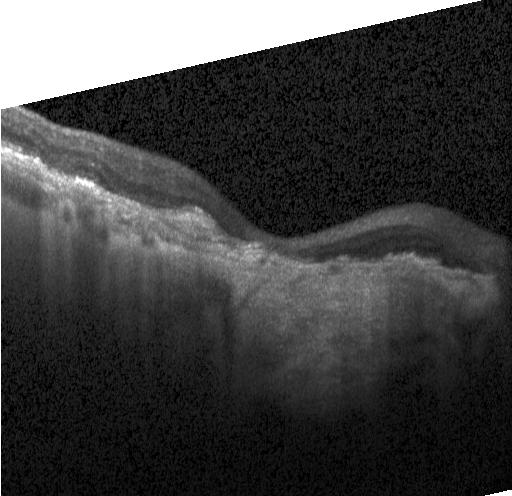

Retinal OCT cross-section — Impression: choroidal neovascularization (CNV).